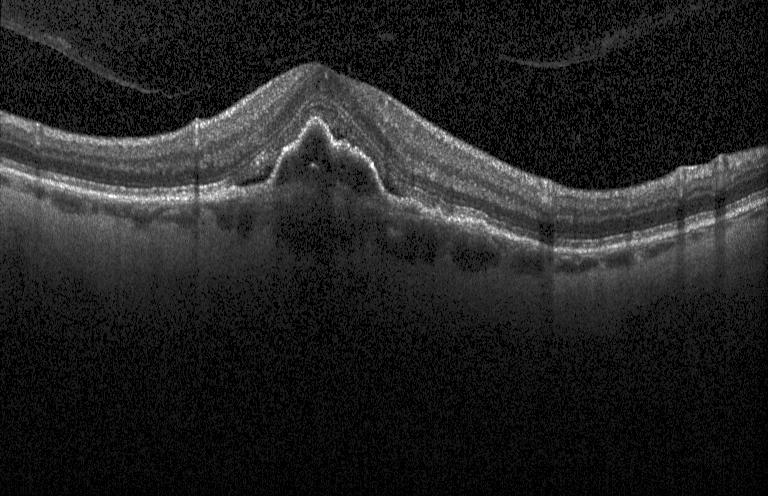
Finding: a choroidal neovascular membrane.